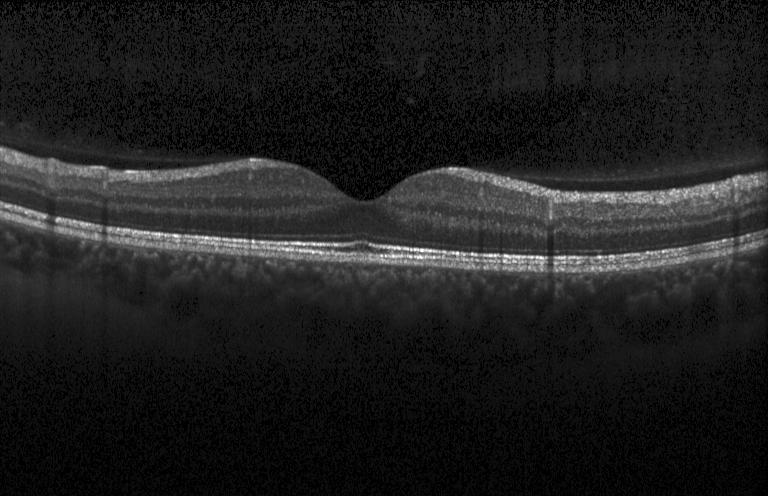 Finding: neither choroidal neovascularization, diabetic macular edema, nor drusen.